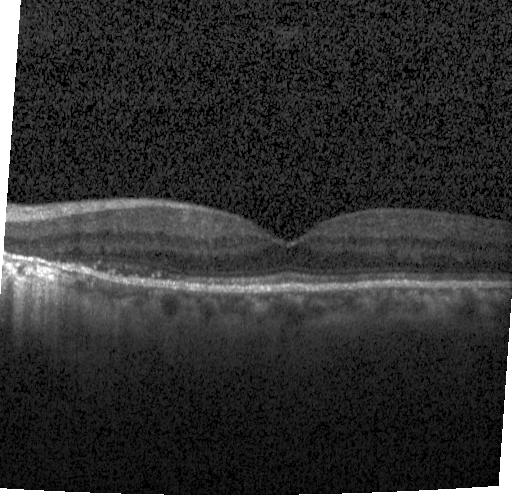 Assessment: no choroidal neovascularization, diabetic macular edema, or drusen.